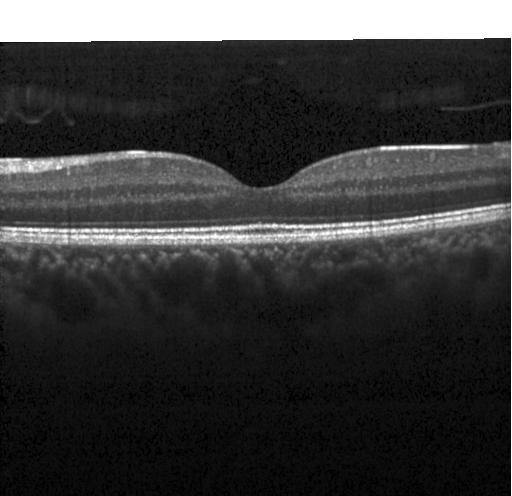 Spectral-domain OCT. OCT line scan. Horizontal scan through the fovea — No evidence of choroidal neovascularization, diabetic macular edema, or drusen.